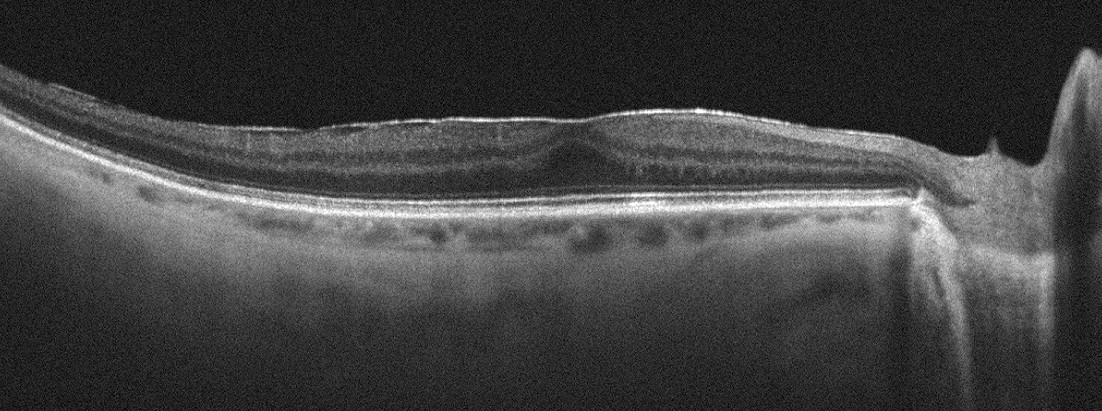

Optical coherence tomography scan. Acquired on an Optovue Avanti RTVue XR.
Epiretinal membrane.